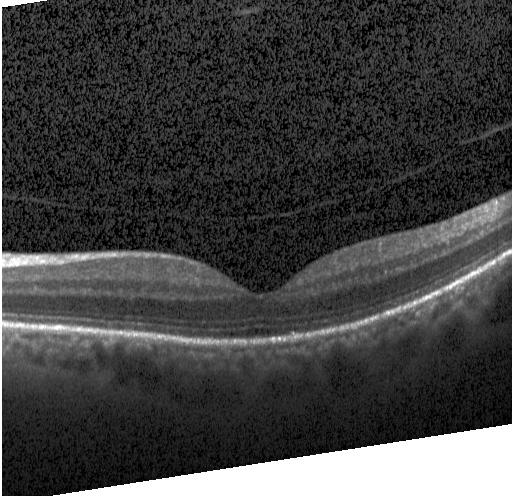
OCT line scan
Dx: no evidence of CNV, DME, or drusen.